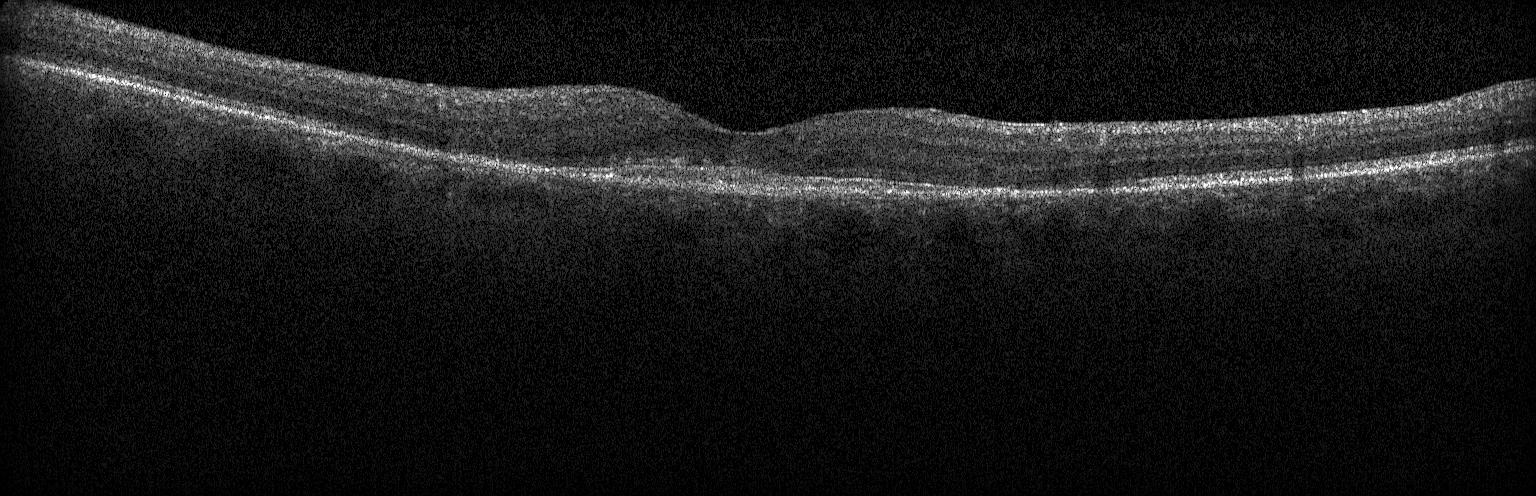 Retinal OCT B-scan
This B-scan demonstrates choroidal neovascularization (CNV).